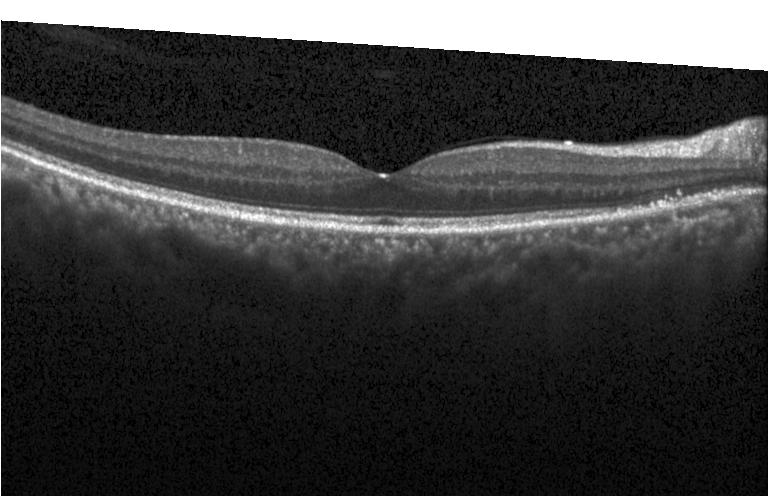

OCT B-scan; horizontal scan through the fovea; instrument: Heidelberg Spectralis. Diagnosis: no CNV, no DME, and no drusen.